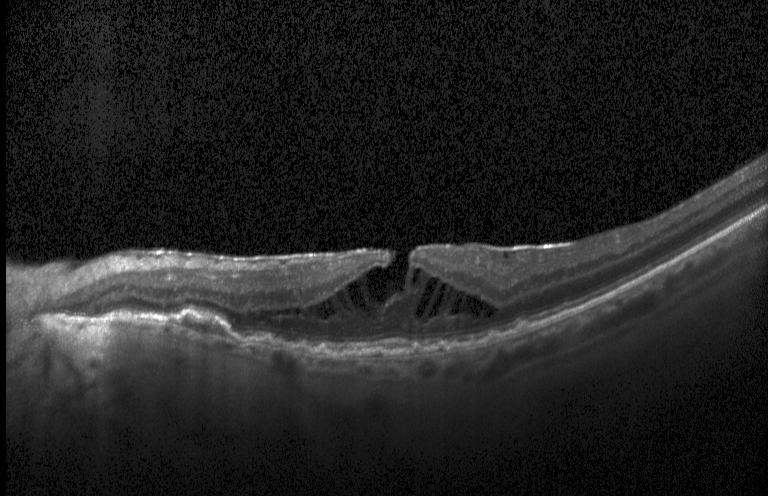
Retinal OCT cross-section showing diabetic macular edema (DME).